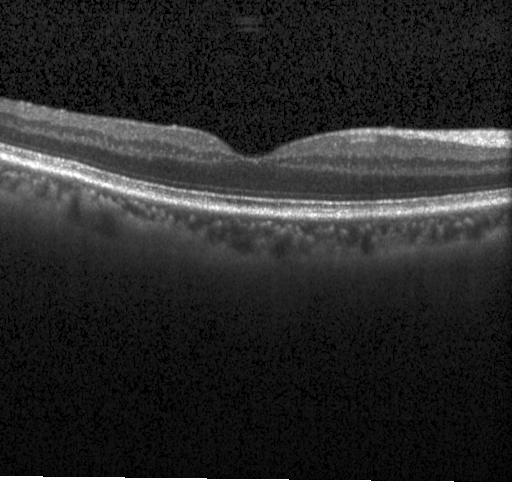

Optical coherence tomography scan; instrument: Heidelberg Spectralis; horizontal scan through the fovea. Finding: no choroidal neovascularization, no diabetic macular edema, and no drusen.